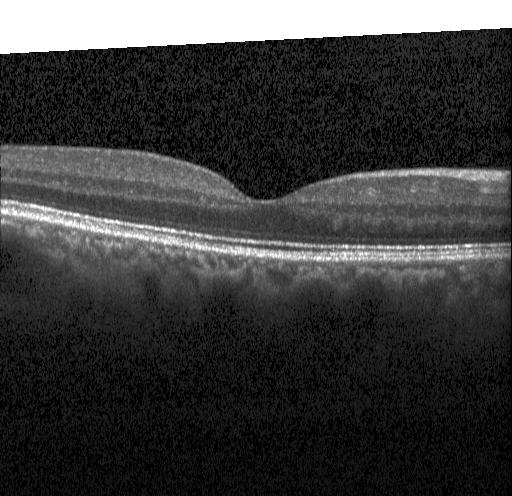

OCT scan showing neither choroidal neovascularization, diabetic macular edema, nor drusen.